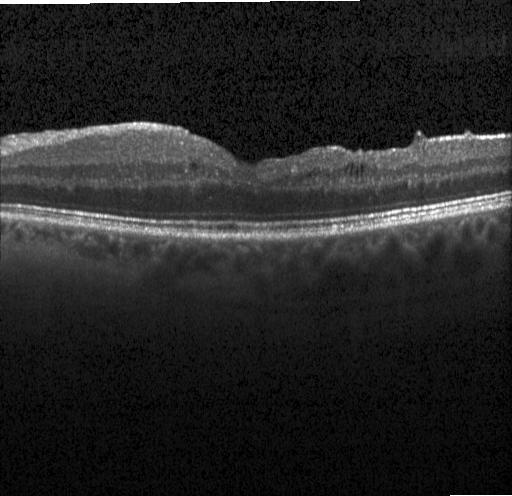 Macular OCT demonstrating DME.